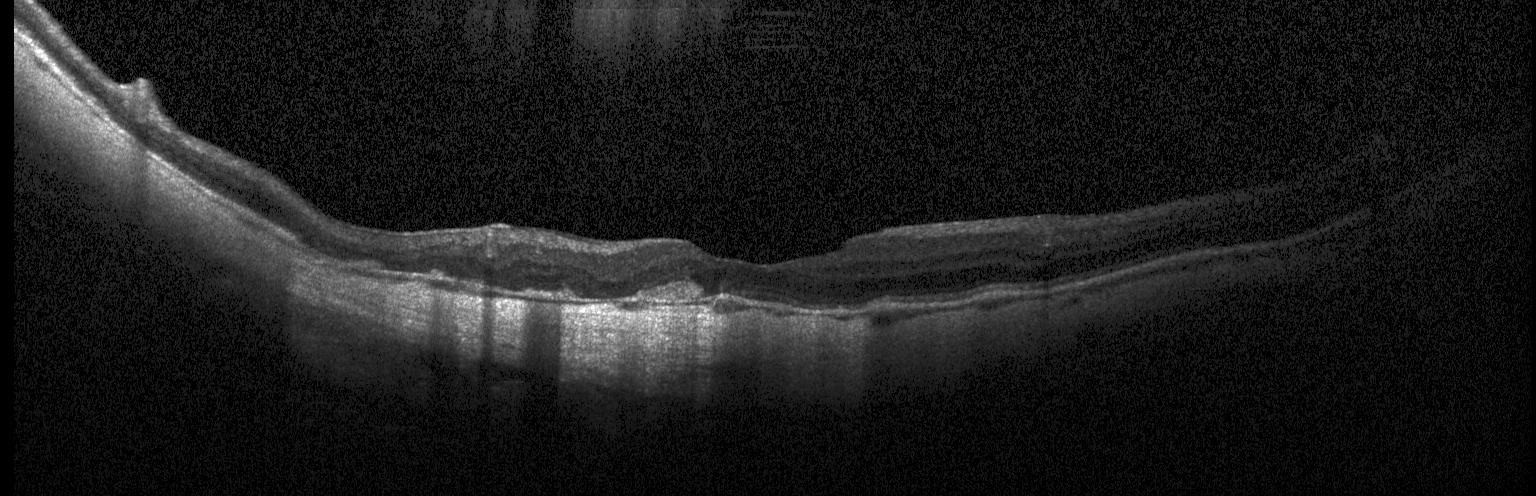

Dx: choroidal neovascularization.